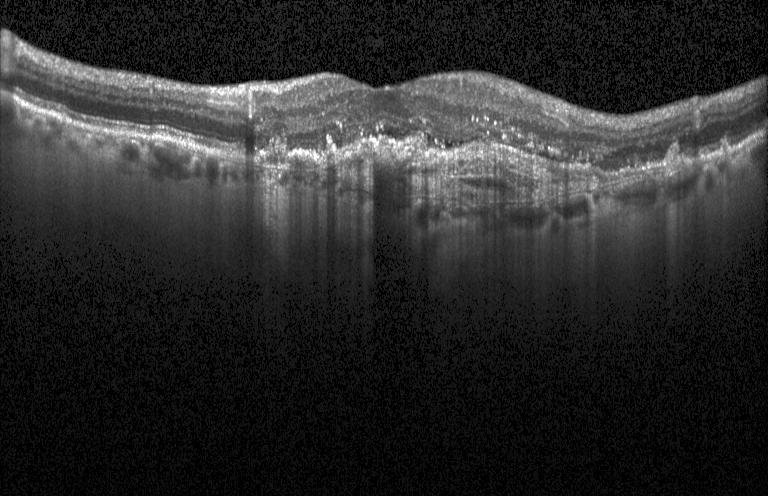 Diagnosis: a choroidal neovascular membrane.